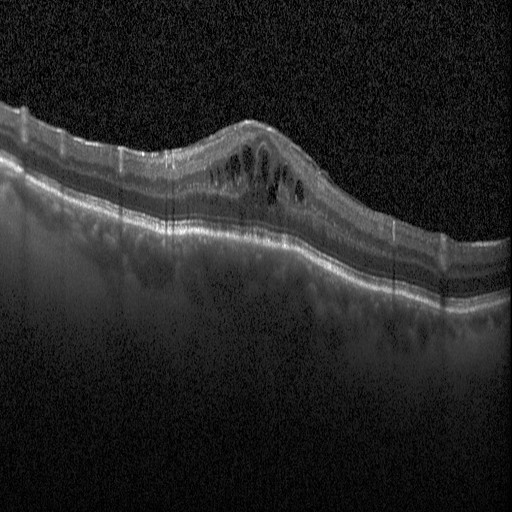 Retinal OCT cross-section. Spectral-domain optical coherence tomography. DME.